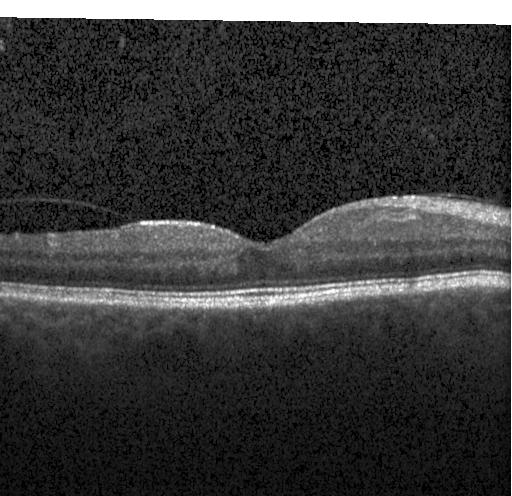 Optical coherence tomography B-scan, Heidelberg Spectralis, macular scan
This B-scan demonstrates no choroidal neovascularization, diabetic macular edema, or drusen.